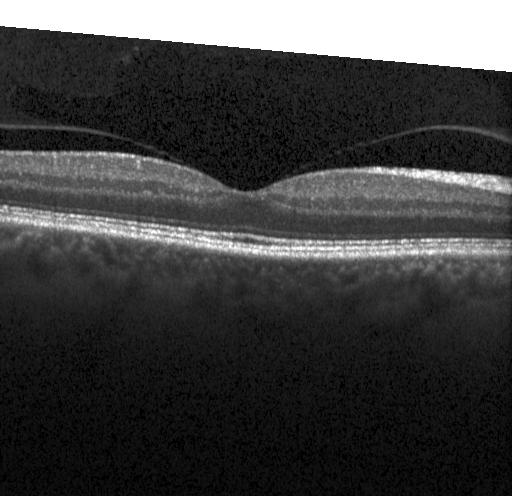 Instrument: Heidelberg Spectralis · optical coherence tomography B-scan.
No choroidal neovascularization, diabetic macular edema, or drusen.